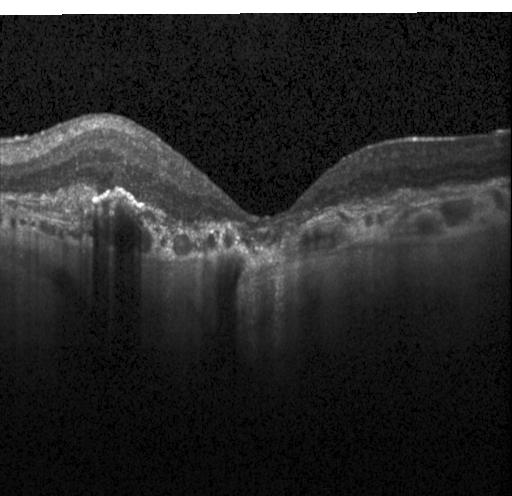 Diagnosis: a choroidal neovascular membrane.